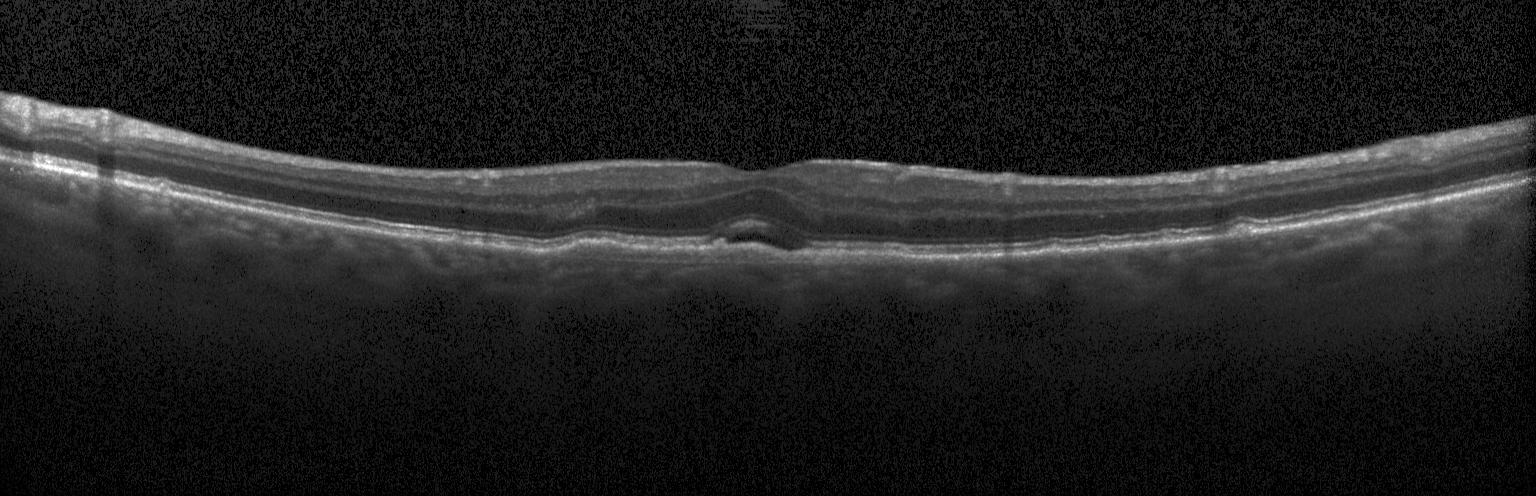 Heidelberg Spectralis OCT system · macular scan · retinal OCT cross-section · SD-OCT.
Impression: choroidal neovascularization.